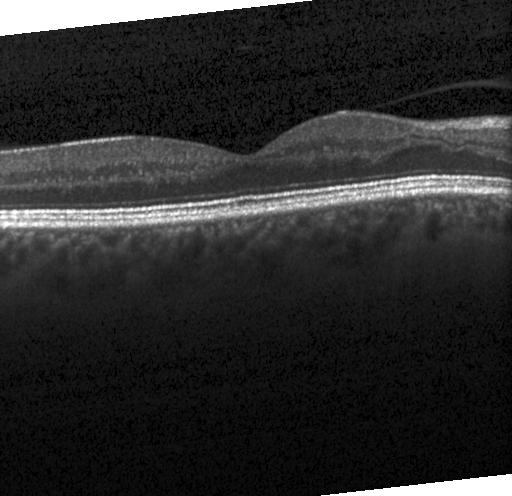
Fovea-centered; retinal OCT cross-section
Macular OCT: no choroidal neovascularization, diabetic macular edema, or drusen.